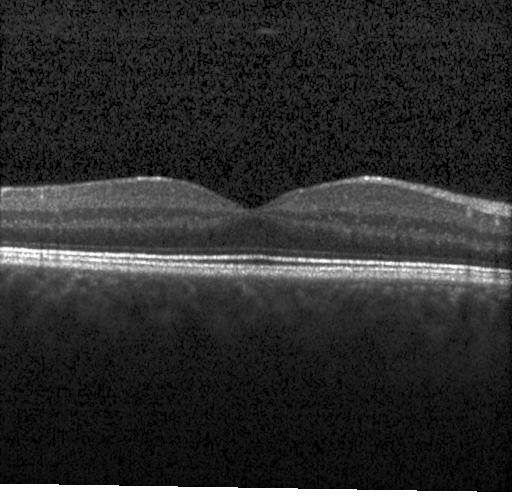 Heidelberg Spectralis OCT system · retinal OCT B-scan
Impression: neither choroidal neovascularization, diabetic macular edema, nor drusen.